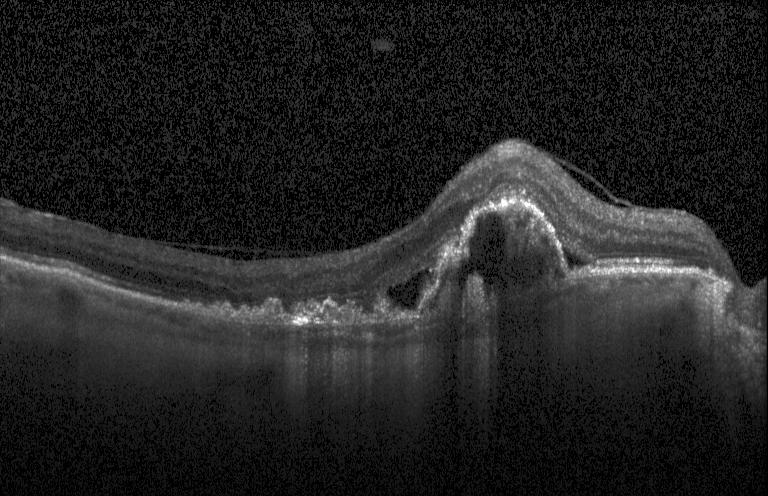 Diagnosis: a choroidal neovascular membrane.